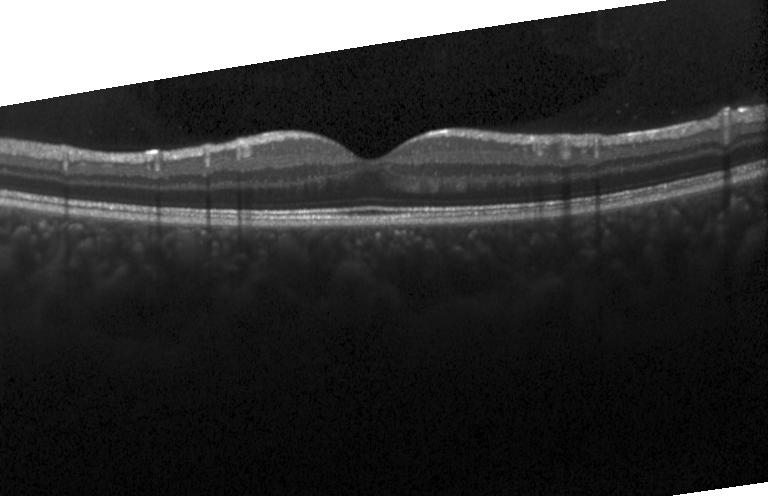 OCT scan showing neither choroidal neovascularization, diabetic macular edema, nor drusen.